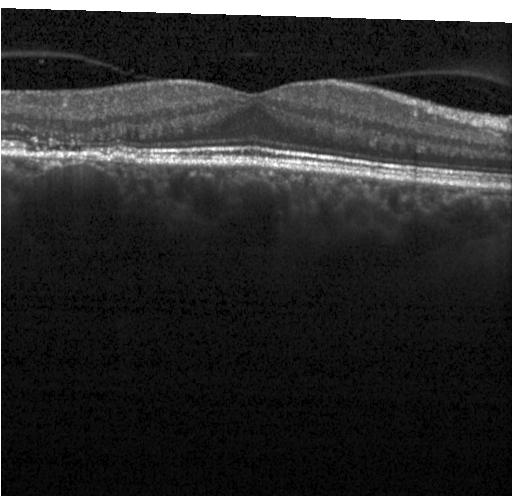
Heidelberg Spectralis OCT system. Macular scan. Retinal OCT cross-section. Spectral-domain optical coherence tomography. Macular OCT: a choroidal neovascular membrane.